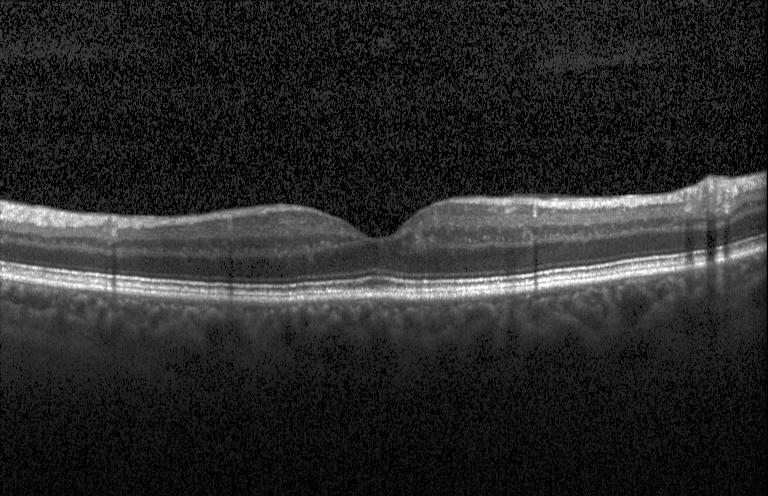 OCT B-scan. Through the macula
Neither choroidal neovascularization, diabetic macular edema, nor drusen.